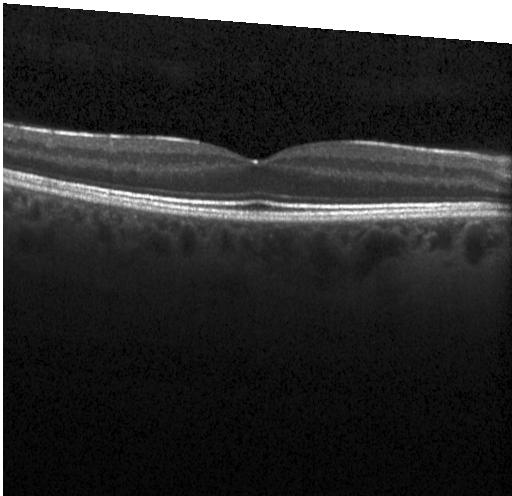 Retinal OCT cross-section; macular scan; Heidelberg Spectralis. OCT finding: no CNV, no DME, and no drusen.